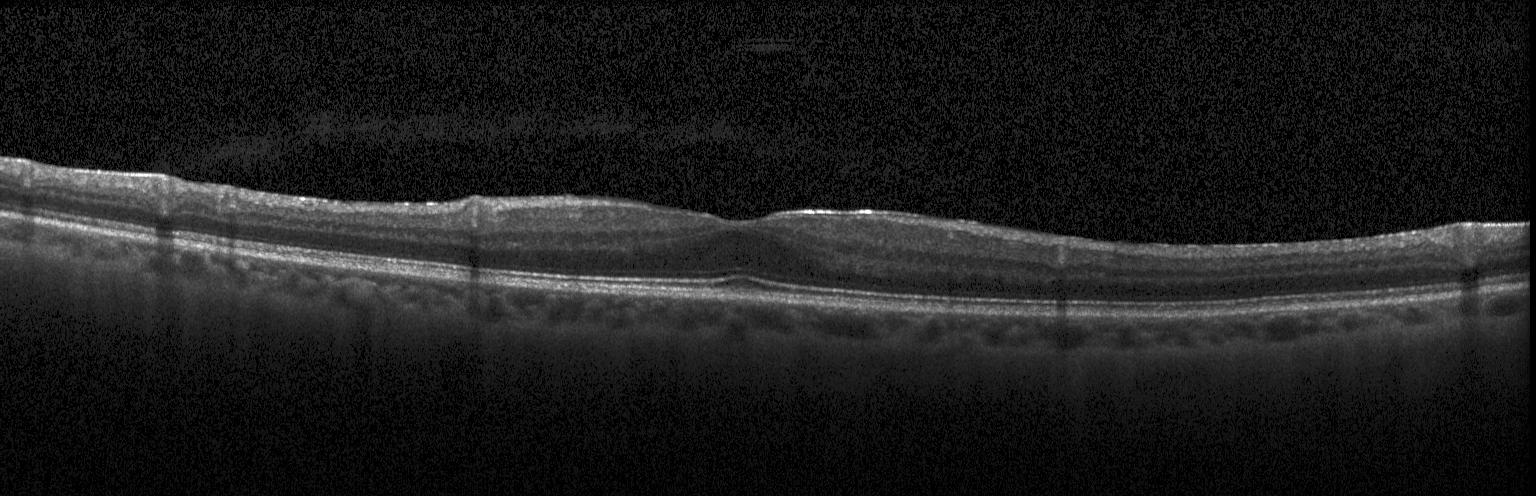 OCT finding: neither choroidal neovascularization, diabetic macular edema, nor drusen.